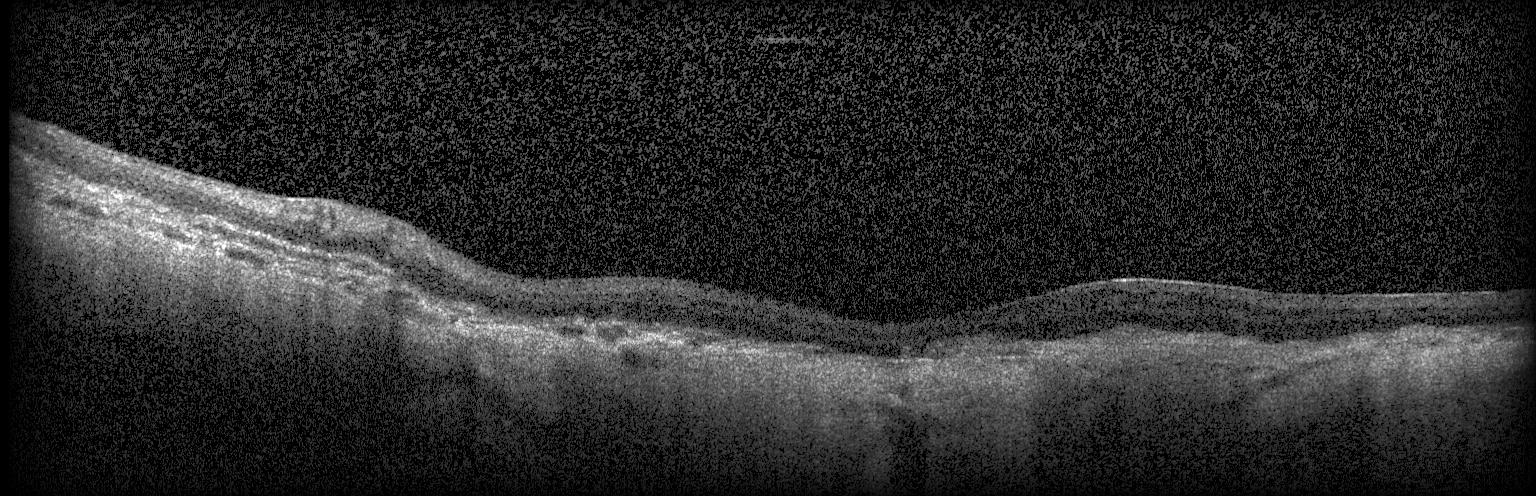

Horizontal scan through the fovea; optical coherence tomography scan
The scan shows choroidal neovascularization (CNV).